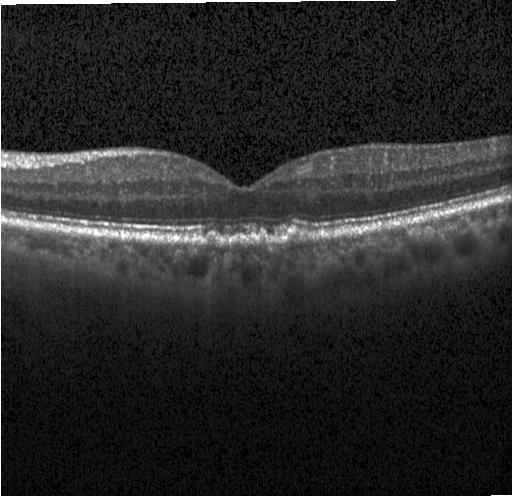
Optical coherence tomography scan · instrument: Heidelberg Spectralis · SD-OCT
Assessment: sub-RPE drusenoid deposits.